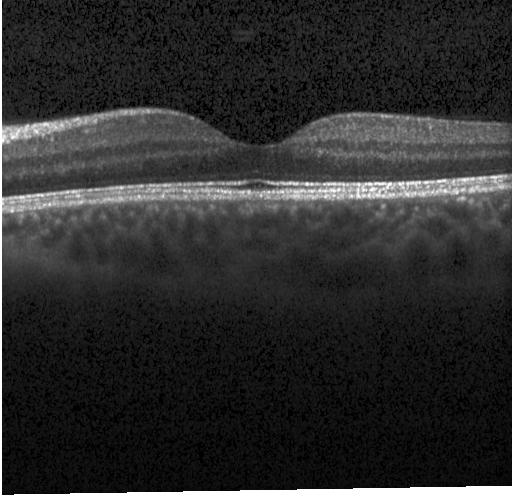 OCT finding: no CNV, no DME, and no drusen.